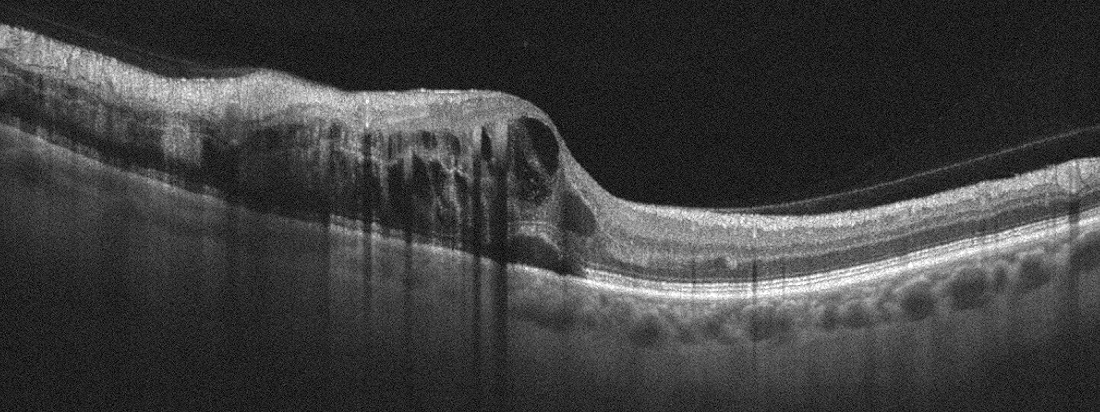
Optical coherence tomography scan. Finding: retinal vein occlusion.